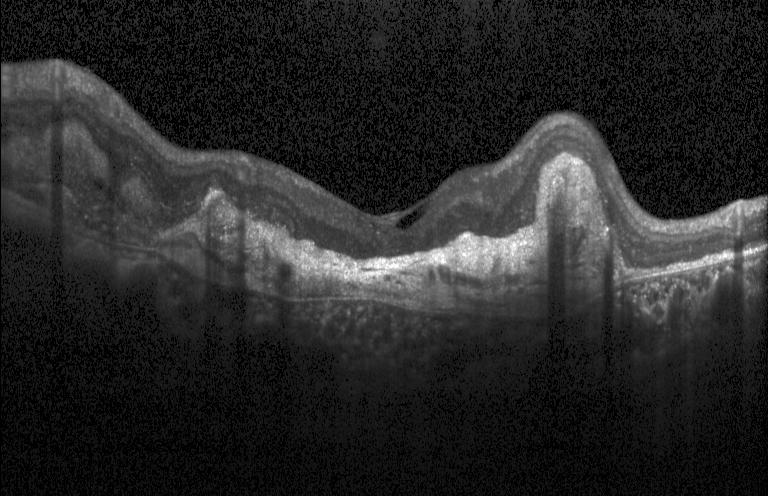

Spectral-domain OCT B-scan: a choroidal neovascular membrane.